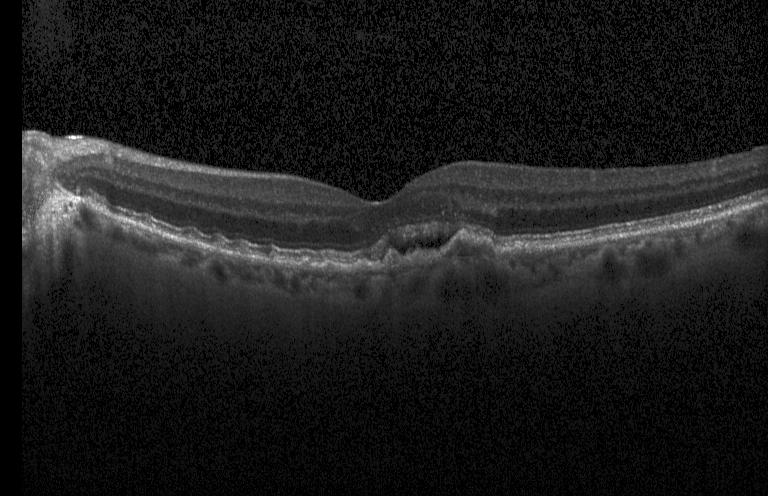 Finding: a choroidal neovascular membrane.